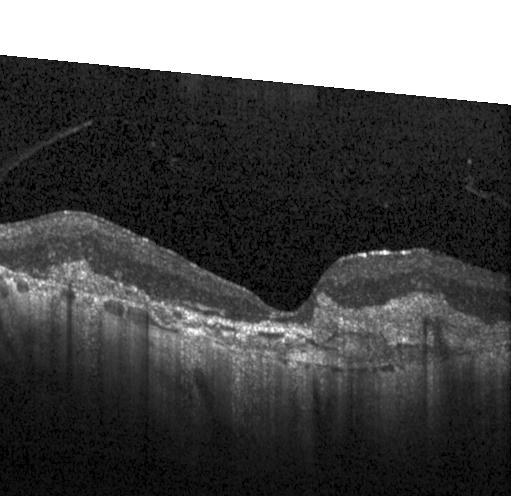 Retinal OCT cross-section — The scan shows CNV.